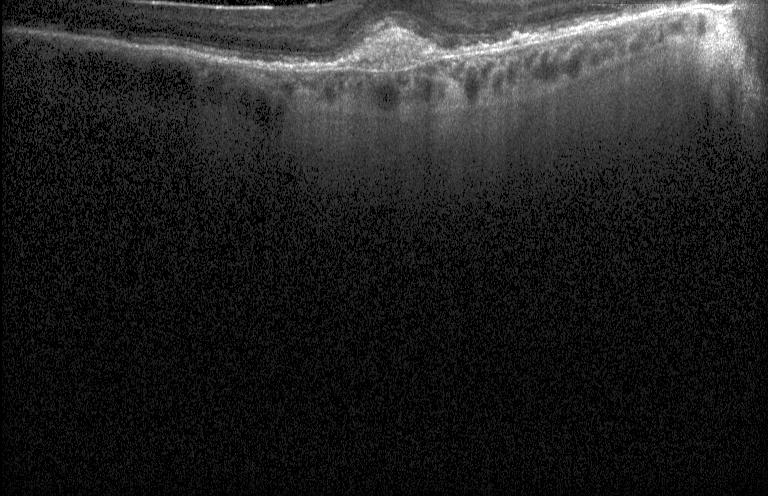

Centered on the fovea; retinal OCT cross-section; SD-OCT; Heidelberg Spectralis OCT system. This B-scan demonstrates CNV.